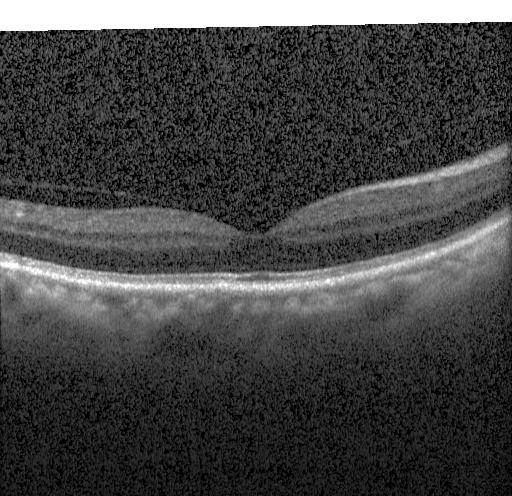
Through the macula. OCT line scan
Macular OCT: no choroidal neovascularization, diabetic macular edema, or drusen.